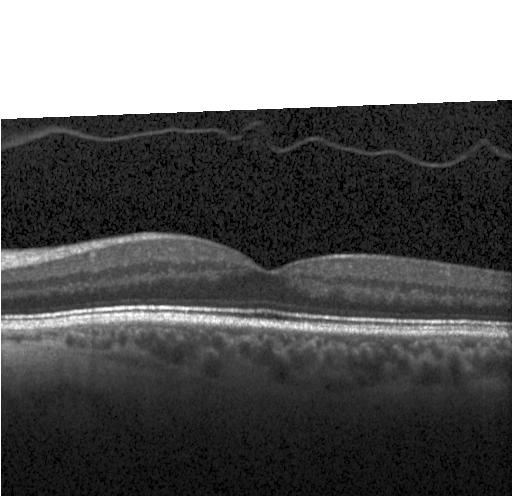
Retinal OCT B-scan; SD-OCT
Assessment: no choroidal neovascularization, diabetic macular edema, or drusen.